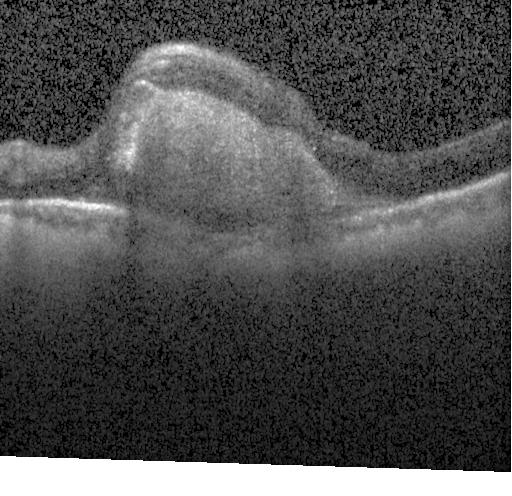
Spectral-domain OCT, optical coherence tomography scan.
CNV.